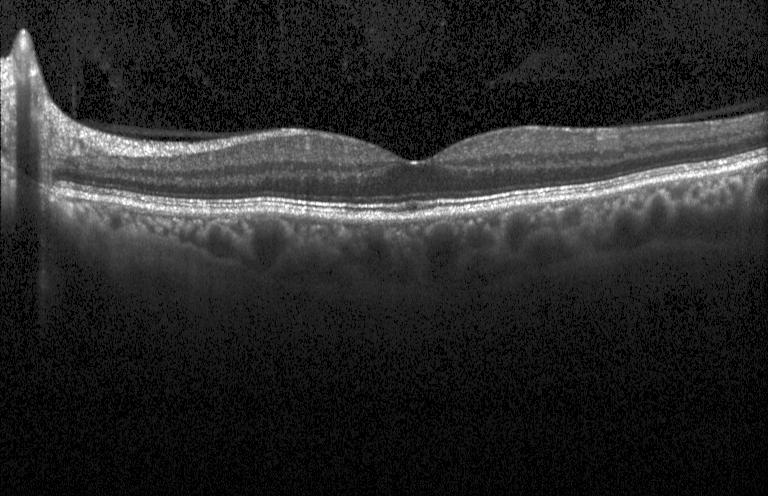 Fovea-centered, spectral-domain OCT, Heidelberg Spectralis, optical coherence tomography B-scan
Finding: neither choroidal neovascularization, diabetic macular edema, nor drusen.